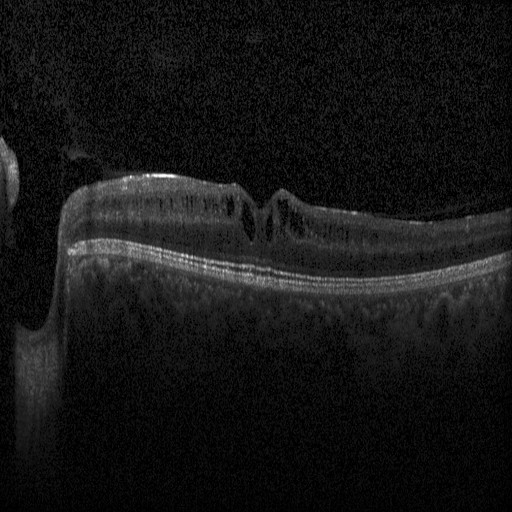

Retinal OCT B-scan · fovea-centered · spectral-domain OCT · acquired on a Heidelberg Spectralis. The scan shows diabetic macular edema.